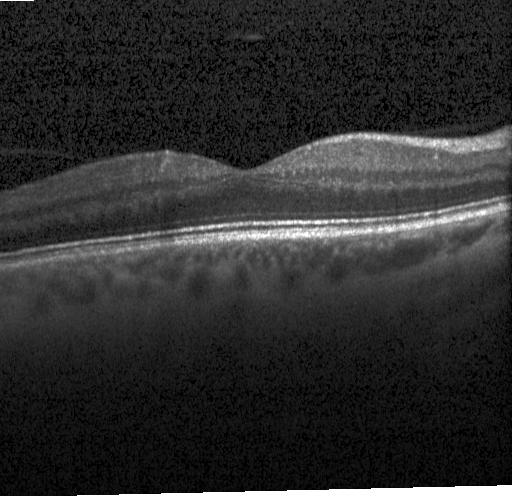
Horizontal scan through the fovea, SD-OCT, optical coherence tomography B-scan, Heidelberg Spectralis — Neither CNV, DME, nor drusen.